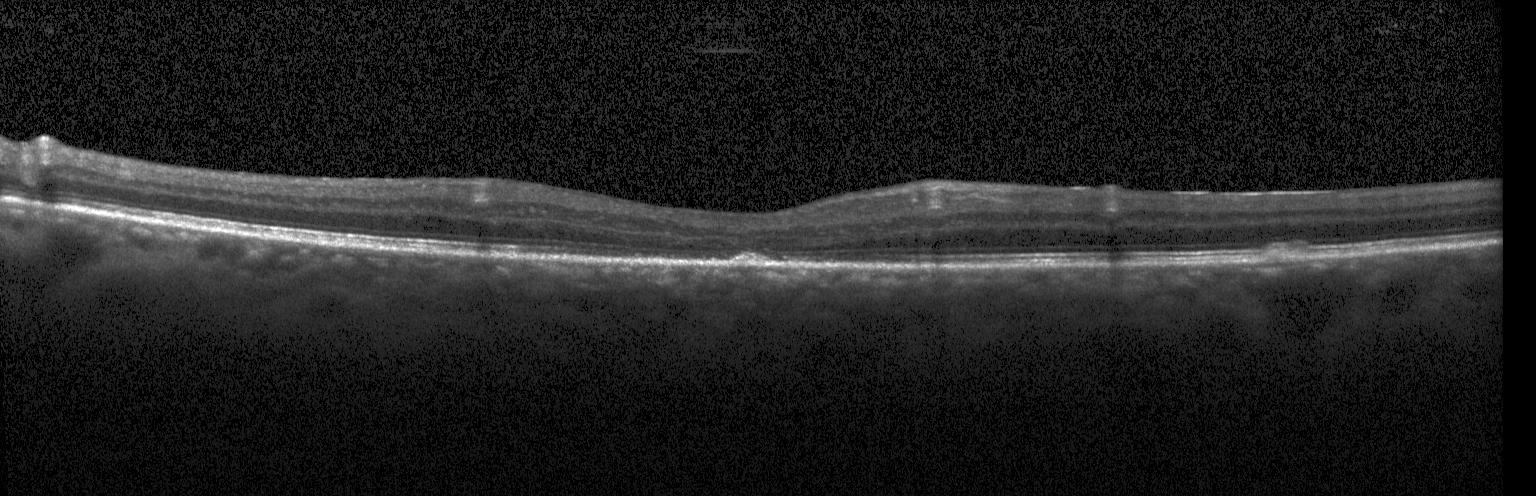
Optical coherence tomography B-scan — Assessment: multiple drusen.